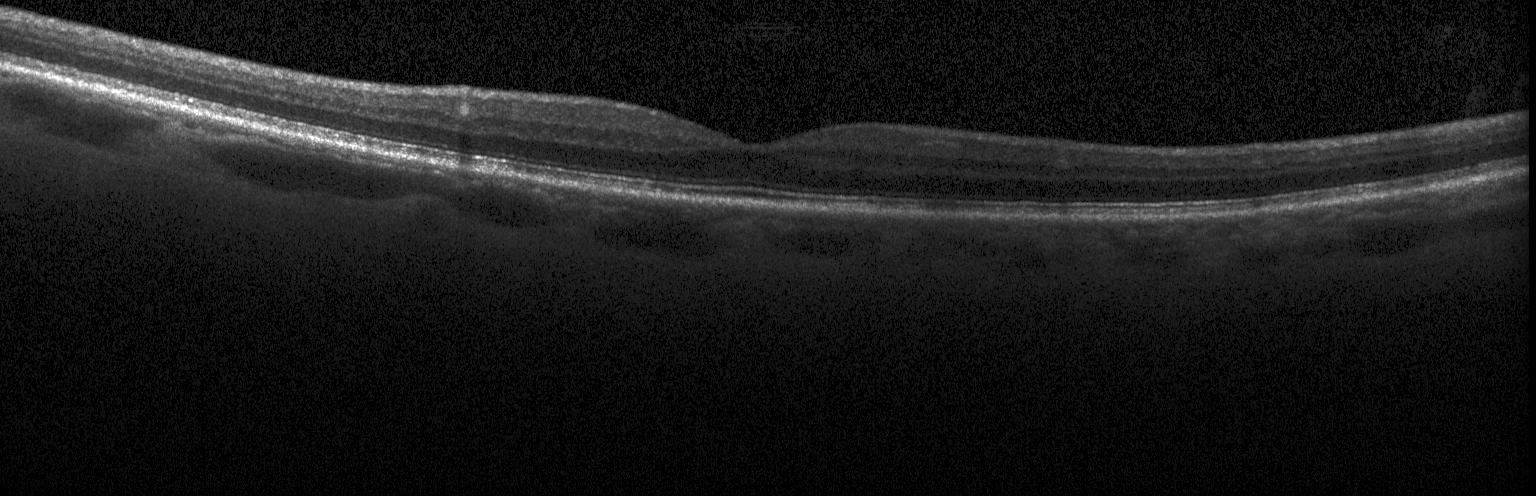

Heidelberg Spectralis, spectral-domain OCT, retinal OCT B-scan. No choroidal neovascularization, no diabetic macular edema, and no drusen.